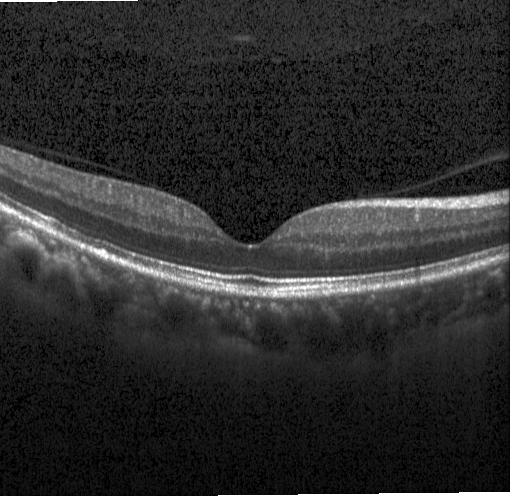
Spectral-domain optical coherence tomography; retinal OCT B-scan; horizontal scan through the fovea; instrument: Heidelberg Spectralis. Neither CNV, DME, nor drusen.